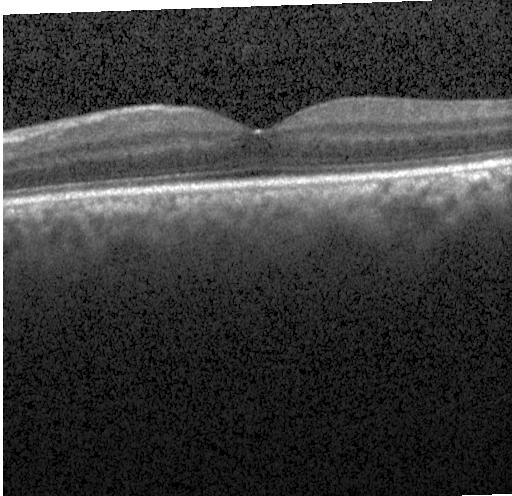 OCT scan showing no CNV, DME, or drusen.